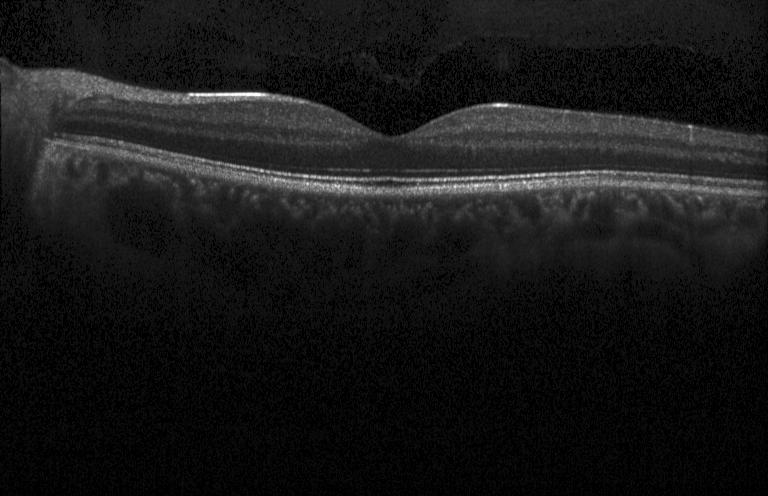 Optical coherence tomography B-scan · macular scan · acquired on a Heidelberg Spectralis
Dx: no choroidal neovascularization, diabetic macular edema, or drusen.